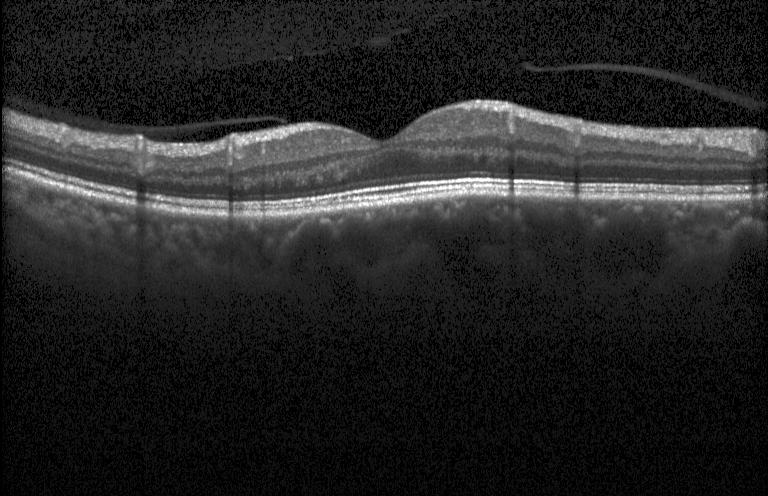

Retinal OCT cross-section. This B-scan demonstrates neither choroidal neovascularization, diabetic macular edema, nor drusen.